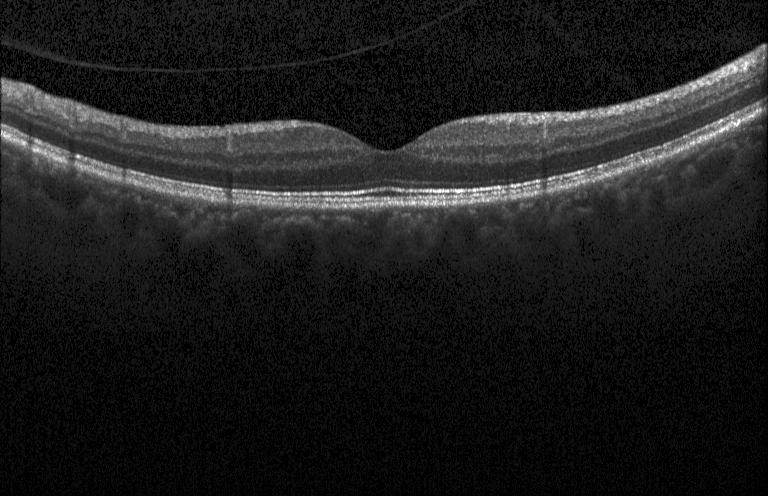
Spectral-domain OCT; OCT line scan. Impression: no evidence of CNV, DME, or drusen.